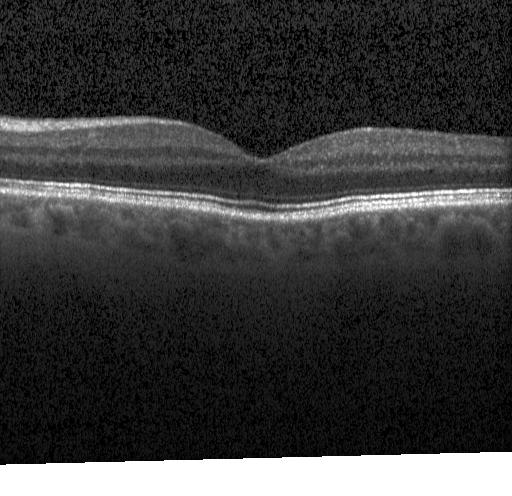 OCT B-scan. Spectral-domain optical coherence tomography — Assessment: neither choroidal neovascularization, diabetic macular edema, nor drusen.